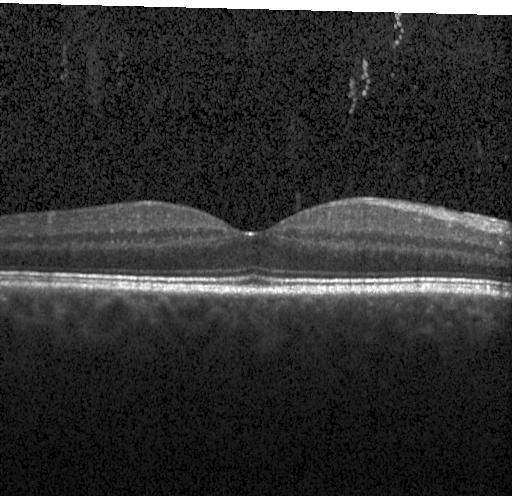
This B-scan demonstrates no evidence of choroidal neovascularization, diabetic macular edema, or drusen.